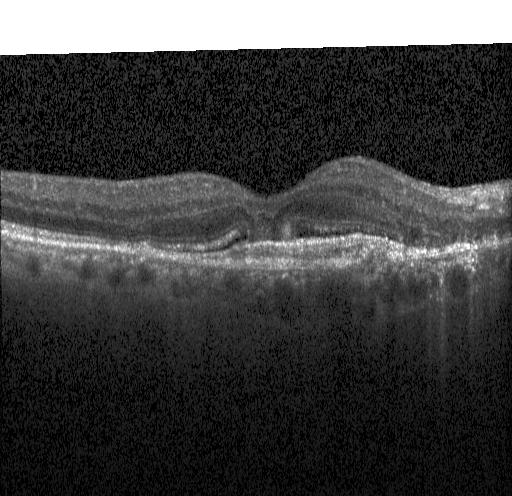
Instrument: Heidelberg Spectralis · retinal OCT cross-section · through the macula — Macular OCT: CNV.